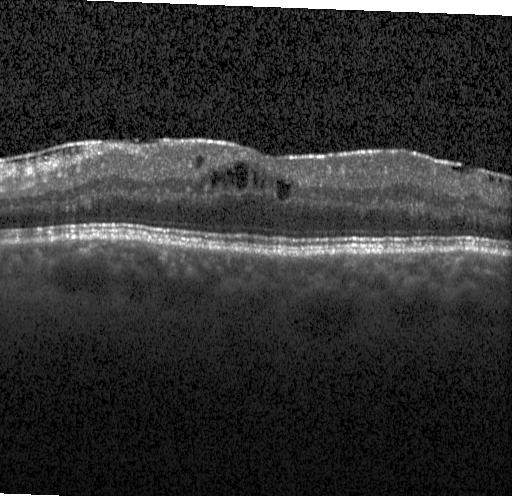

Retinal OCT cross-section. Assessment: diabetic macular edema (DME).